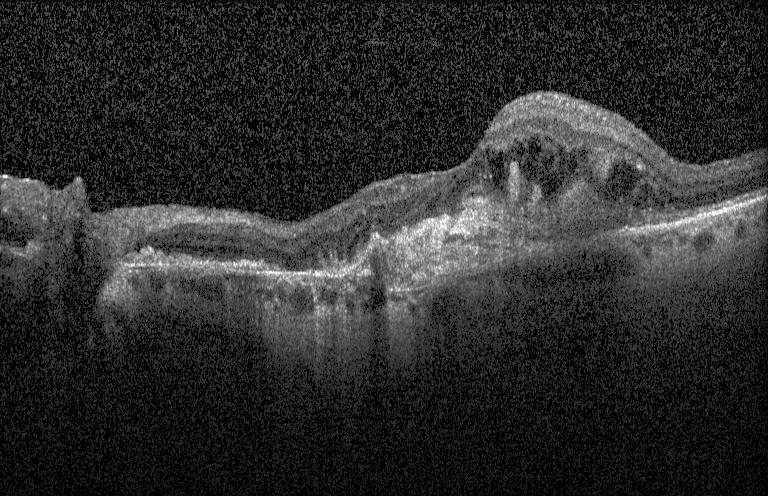 Fovea-centered; OCT line scan; SD-OCT; instrument: Heidelberg Spectralis
Diagnosis: a choroidal neovascular membrane.